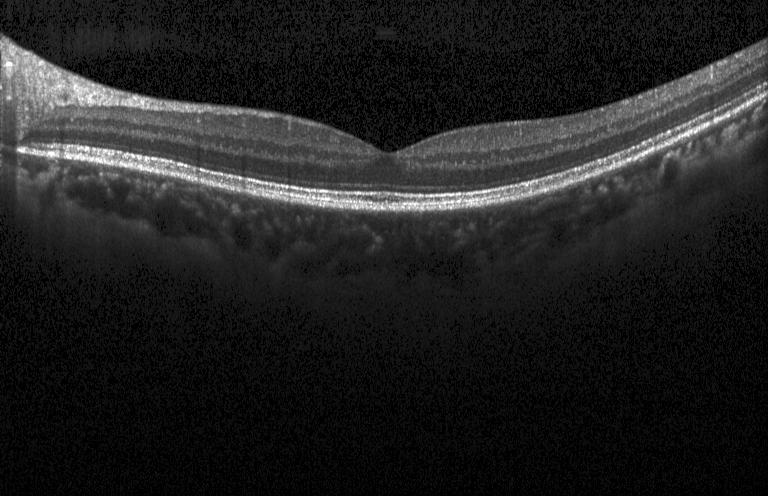
Fovea-centered · retinal OCT B-scan.
Finding: no evidence of CNV, DME, or drusen.